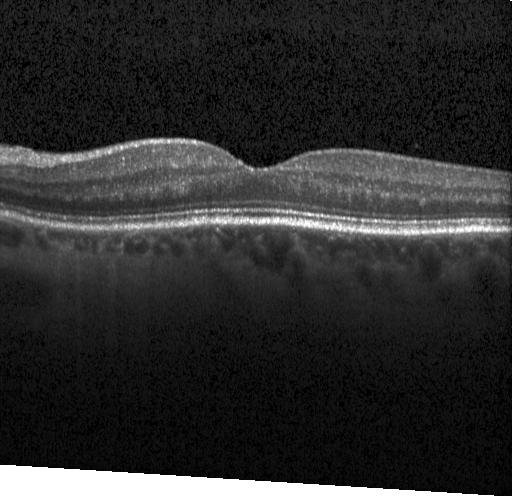

Macular scan · optical coherence tomography scan — Diagnosis: no evidence of choroidal neovascularization, diabetic macular edema, or drusen.